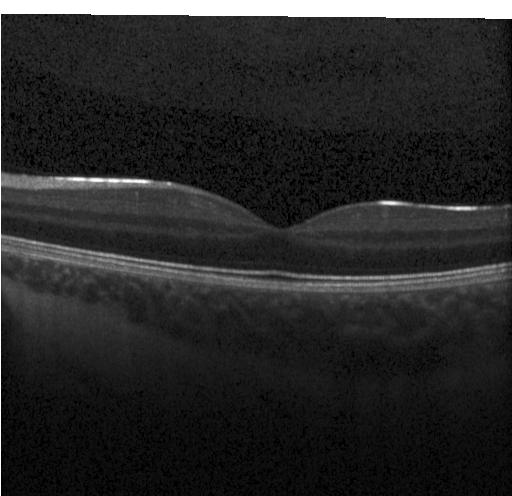 Impression: neither CNV, DME, nor drusen.